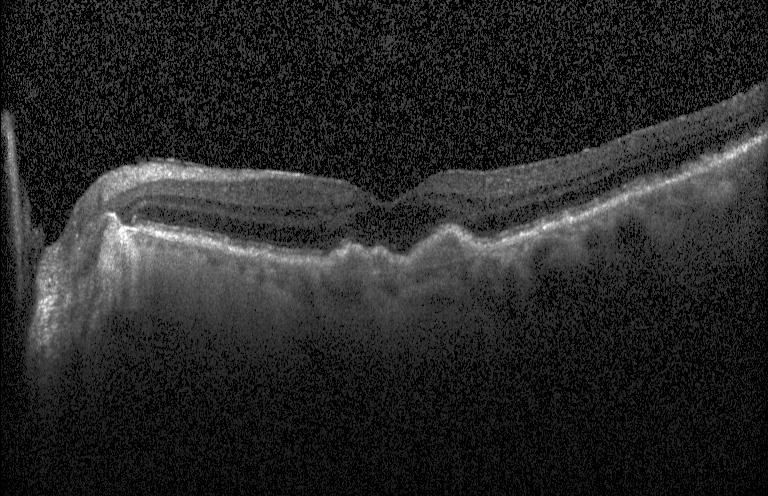 OCT B-scan · Heidelberg Spectralis — This B-scan demonstrates a choroidal neovascular membrane.